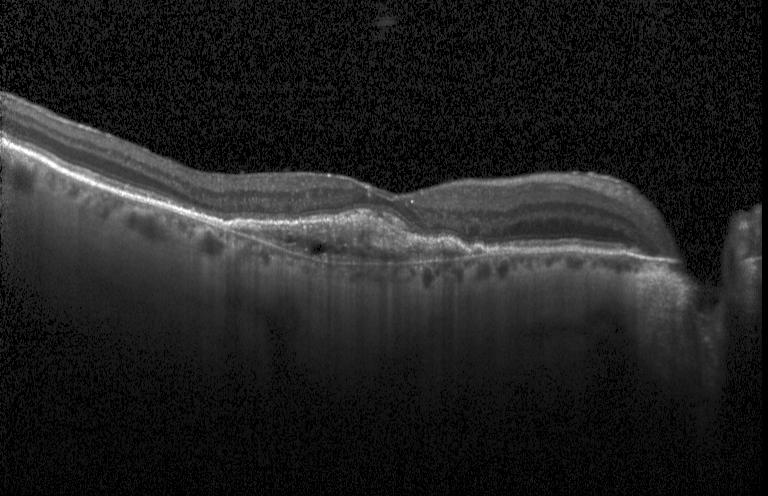

OCT scan showing a choroidal neovascular membrane.